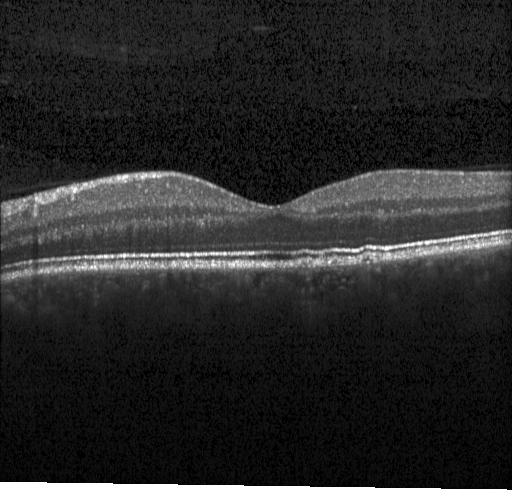
Through the macula, OCT line scan
This B-scan demonstrates drusen.